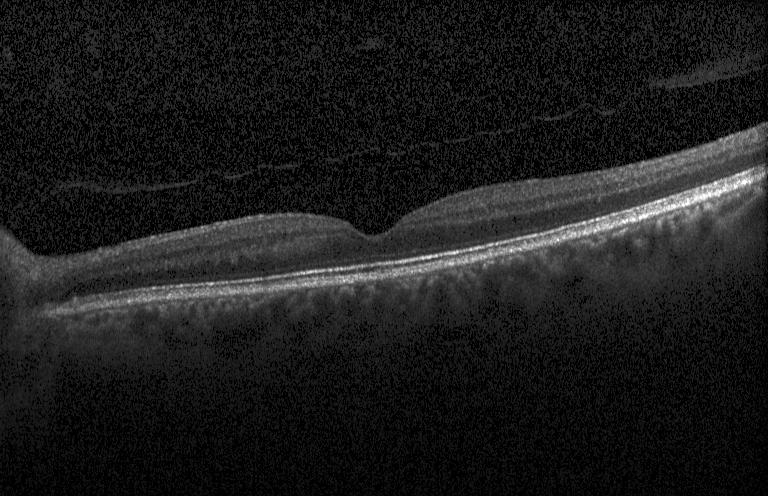 The scan shows no CNV, no DME, and no drusen.